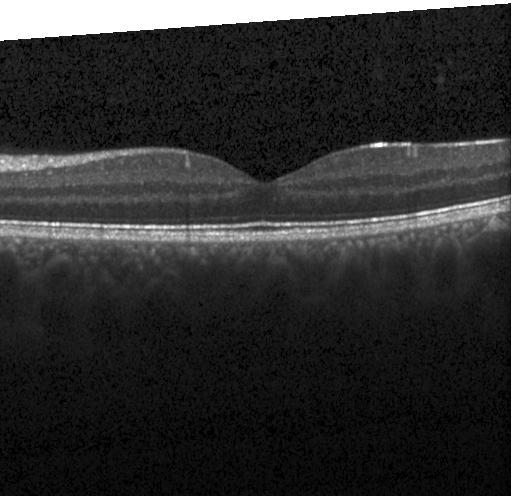
Optical coherence tomography B-scan, spectral-domain optical coherence tomography, horizontal scan through the fovea
This B-scan demonstrates no evidence of CNV, DME, or drusen.